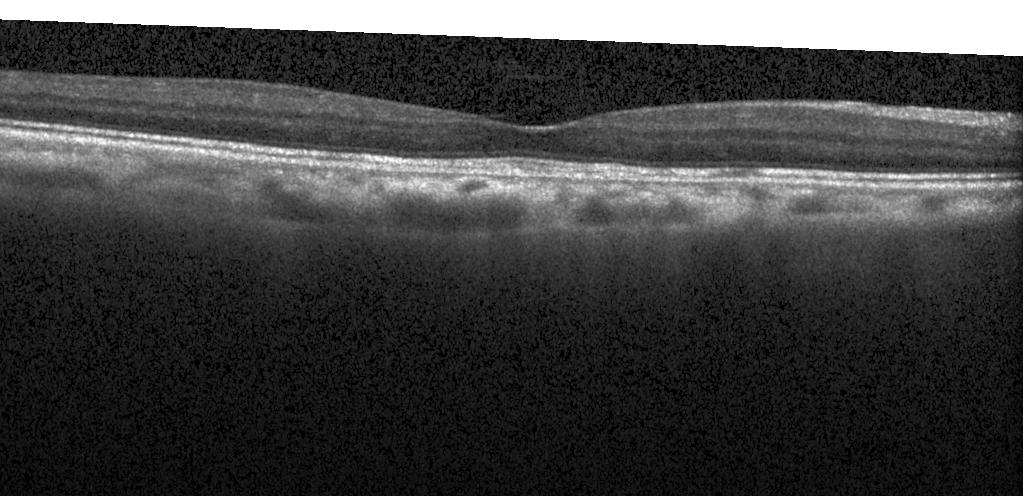

Retinal OCT cross-section showing no choroidal neovascularization, no diabetic macular edema, and no drusen.